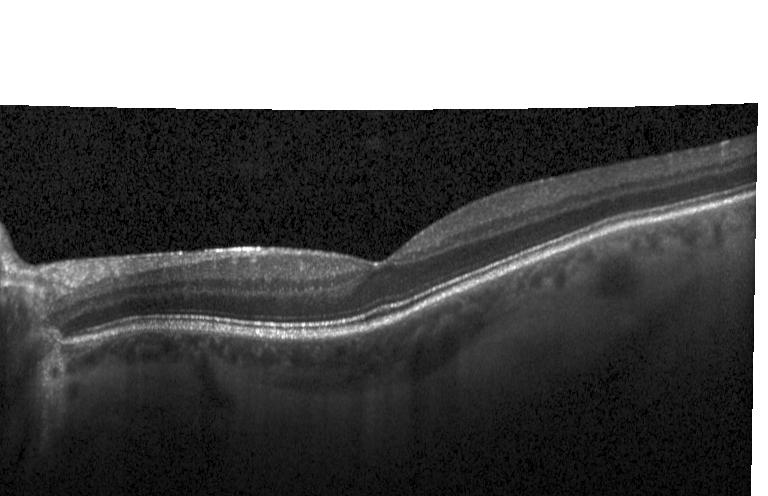
OCT line scan, spectral-domain optical coherence tomography
Dx: neither CNV, DME, nor drusen.